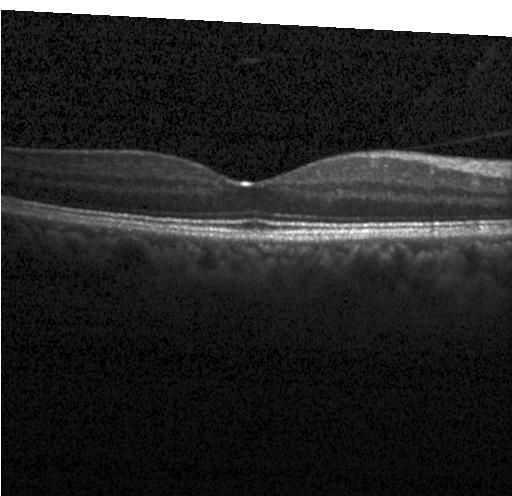
Retinal OCT cross-section. OCT finding: no choroidal neovascularization, no diabetic macular edema, and no drusen.